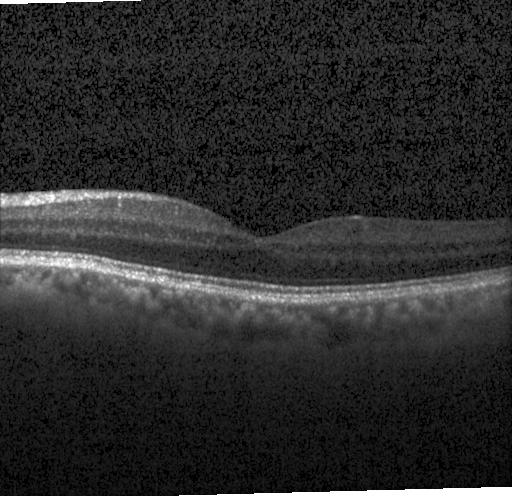 OCT line scan, centered on the fovea.
Impression: neither choroidal neovascularization, diabetic macular edema, nor drusen.